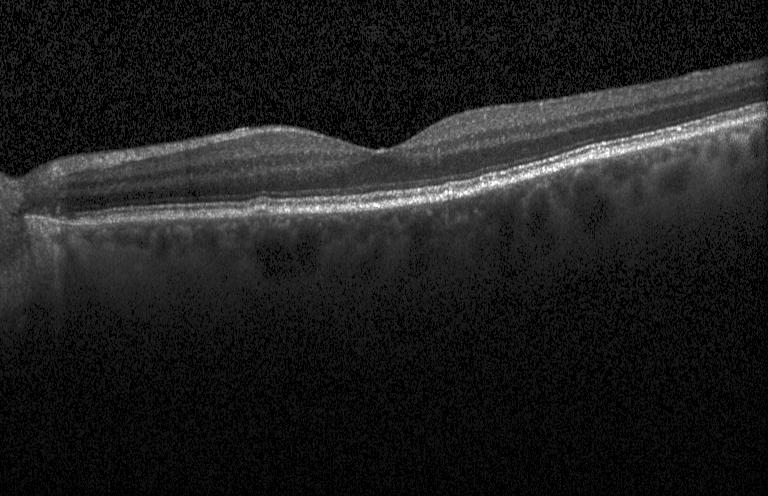 Optical coherence tomography B-scan — Sub-RPE drusenoid deposits.